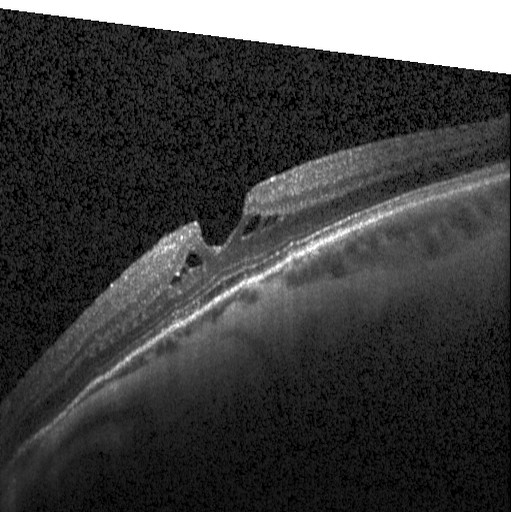 Optical coherence tomography B-scan, macular scan
Diagnosis: diabetic macular edema.